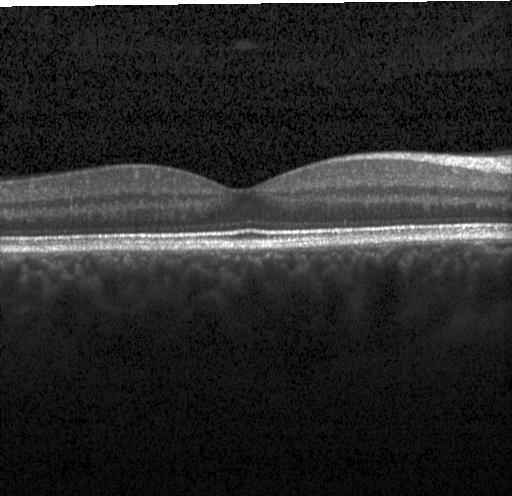

Macular OCT demonstrating neither CNV, DME, nor drusen.